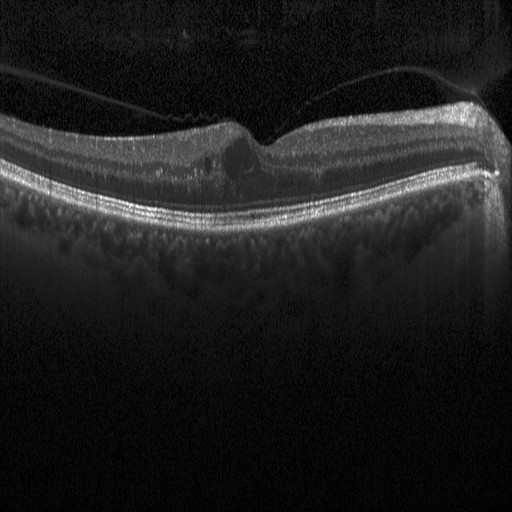 Macular OCT: DME.